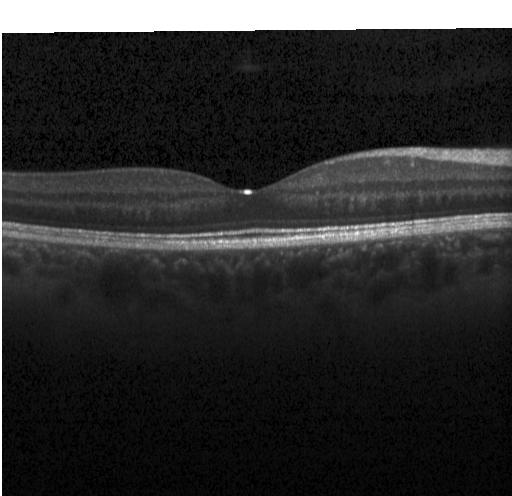
Optical coherence tomography B-scan. Finding: neither choroidal neovascularization, diabetic macular edema, nor drusen.